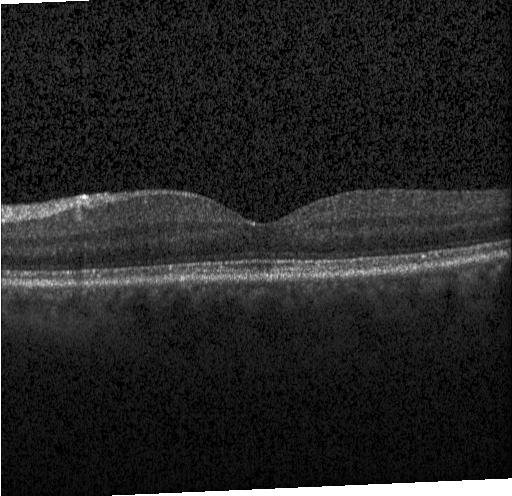
Optical coherence tomography B-scan; instrument: Heidelberg Spectralis. Assessment: no choroidal neovascularization, diabetic macular edema, or drusen.